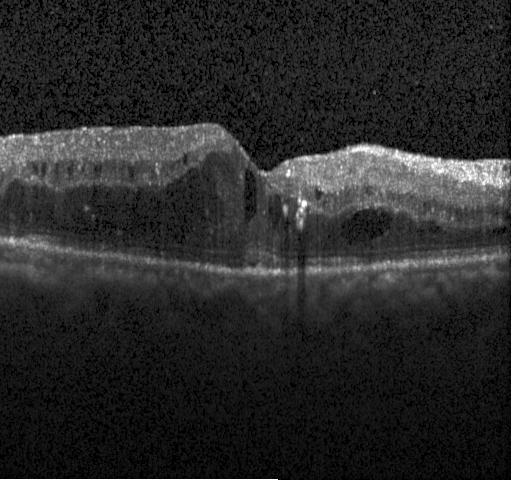

Spectral-domain OCT; OCT line scan; horizontal scan through the fovea; instrument: Heidelberg Spectralis — This B-scan demonstrates diabetic macular edema (DME).